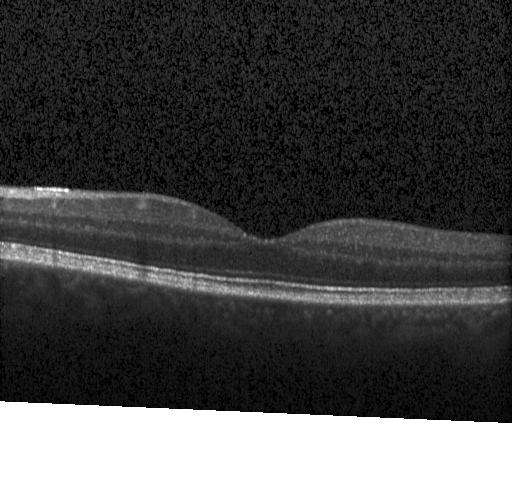 Optical coherence tomography scan.
Finding: no evidence of choroidal neovascularization, diabetic macular edema, or drusen.